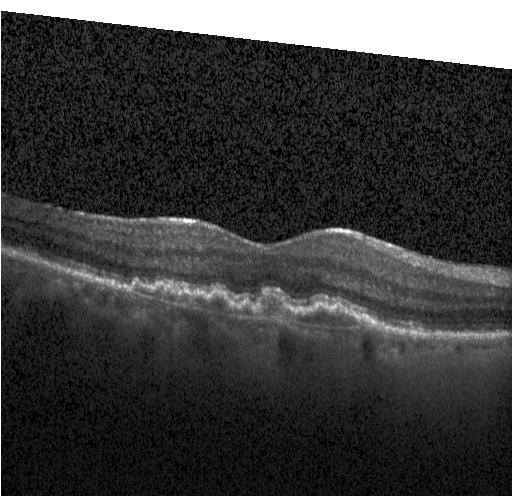

Instrument: Heidelberg Spectralis, macular scan, optical coherence tomography scan.
Dx: choroidal neovascularization.